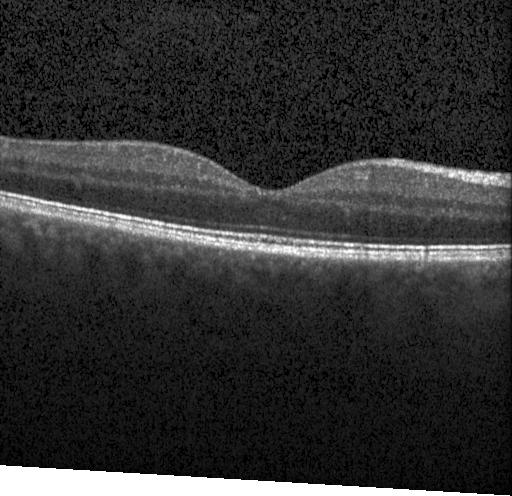
This B-scan demonstrates neither choroidal neovascularization, diabetic macular edema, nor drusen.